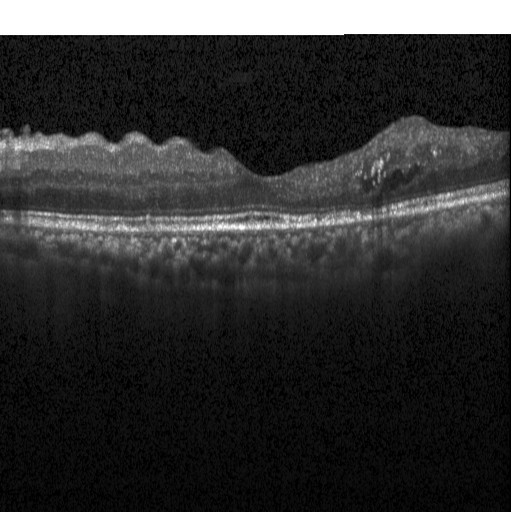
Fovea-centered · retinal OCT cross-section · spectral-domain optical coherence tomography
Macular OCT: diabetic macular edema (DME).